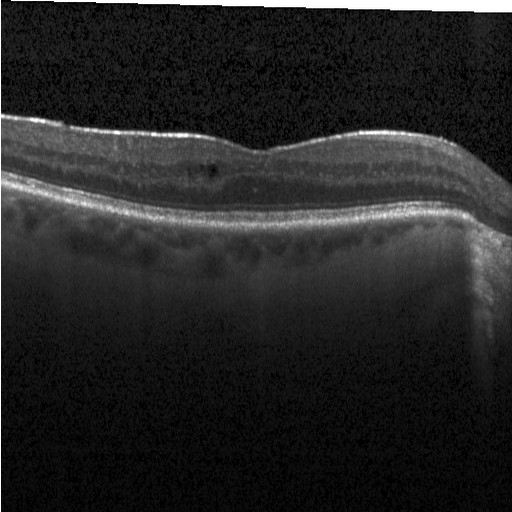

Through the macula; retinal OCT B-scan; spectral-domain OCT; instrument: Heidelberg Spectralis. Impression: diabetic macular edema.